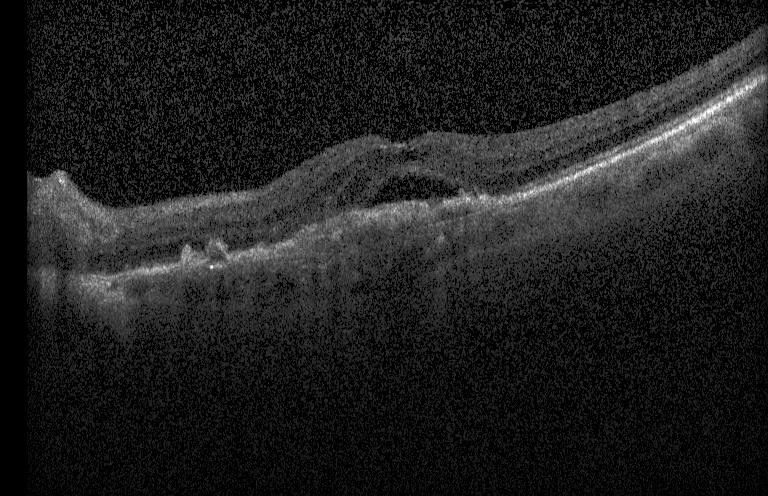

Horizontal scan through the fovea · retinal OCT B-scan · spectral-domain OCT.
Assessment: choroidal neovascularization.